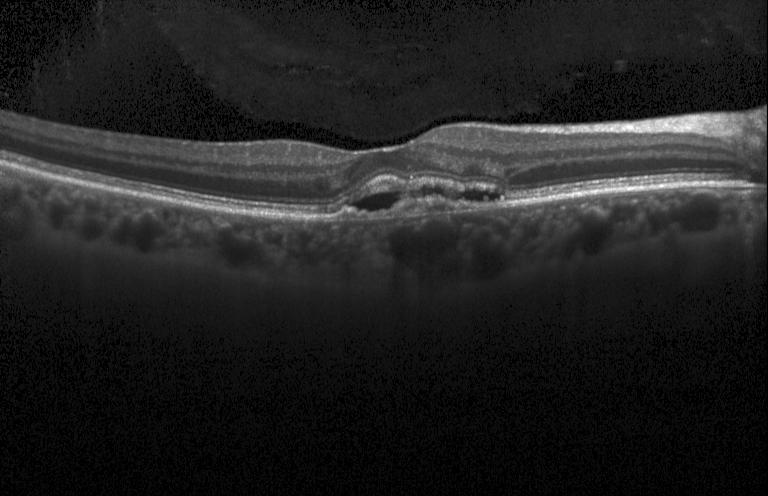 Spectral-domain OCT B-scan: a choroidal neovascular membrane.